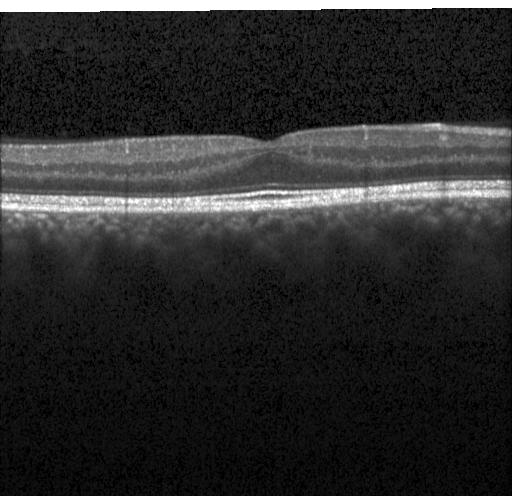
Retinal OCT cross-section.
Finding: no choroidal neovascularization, no diabetic macular edema, and no drusen.